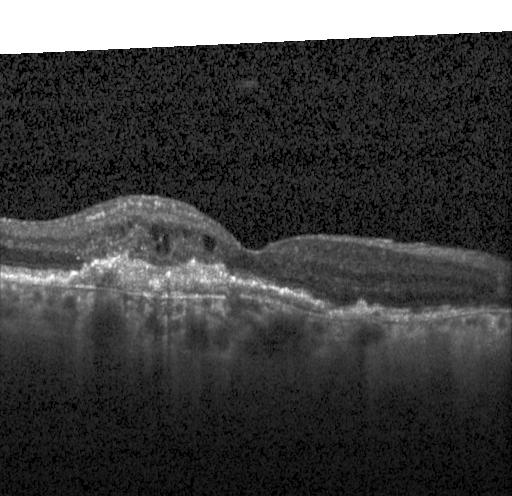
This B-scan demonstrates choroidal neovascularization.